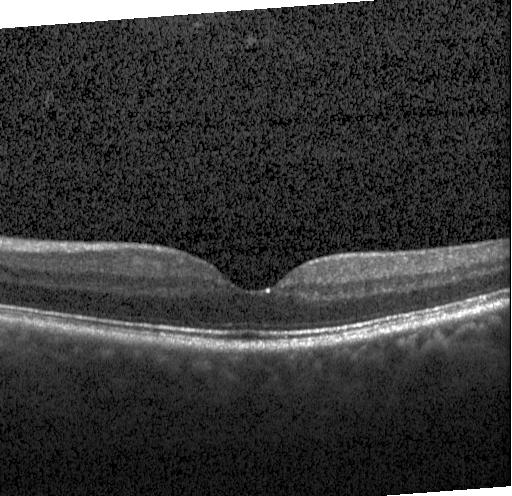 SD-OCT. Optical coherence tomography scan. Acquired on a Heidelberg Spectralis.
Neither choroidal neovascularization, diabetic macular edema, nor drusen.